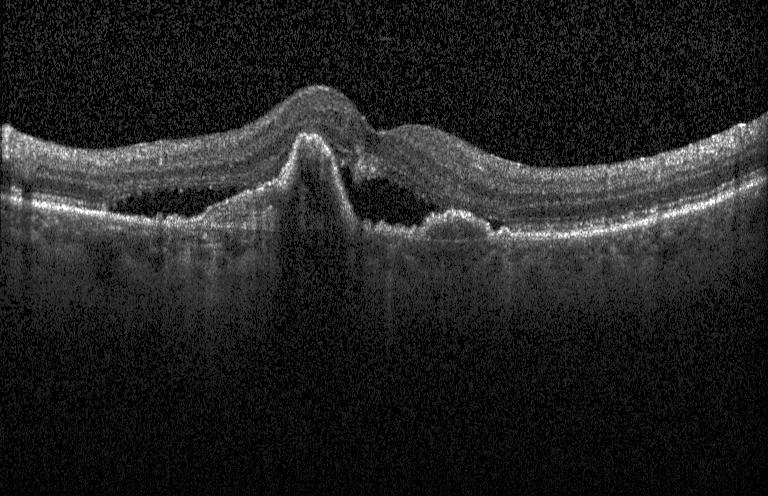

Optical coherence tomography scan — CNV.